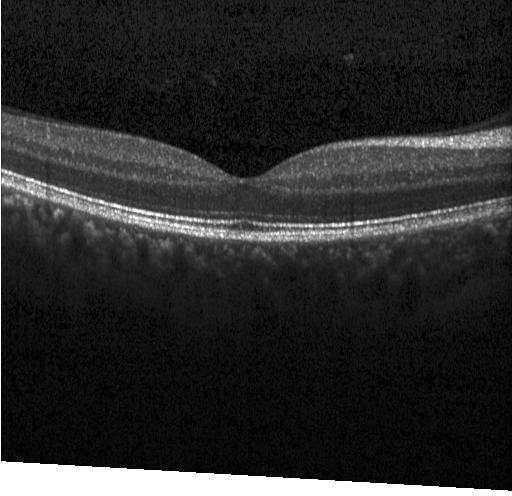
Retinal OCT B-scan, instrument: Heidelberg Spectralis, horizontal scan through the fovea — Finding: no choroidal neovascularization, diabetic macular edema, or drusen.